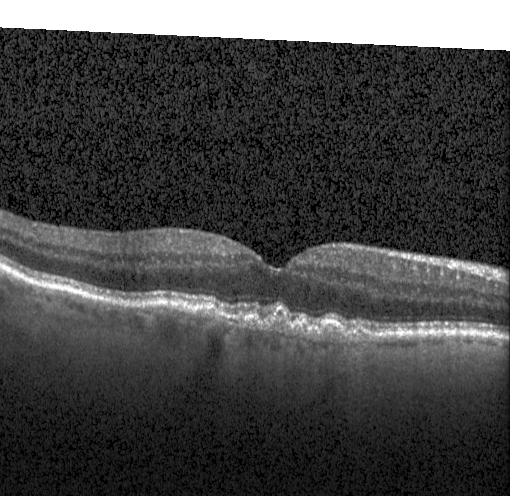
Heidelberg Spectralis OCT system. Optical coherence tomography B-scan
This B-scan demonstrates sub-RPE drusenoid deposits.